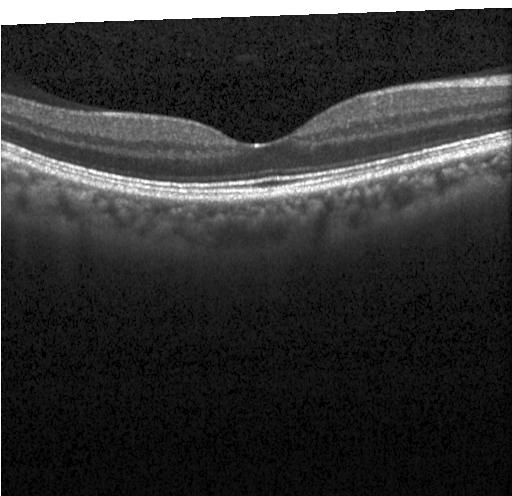 Optical coherence tomography B-scan
Assessment: no evidence of CNV, DME, or drusen.